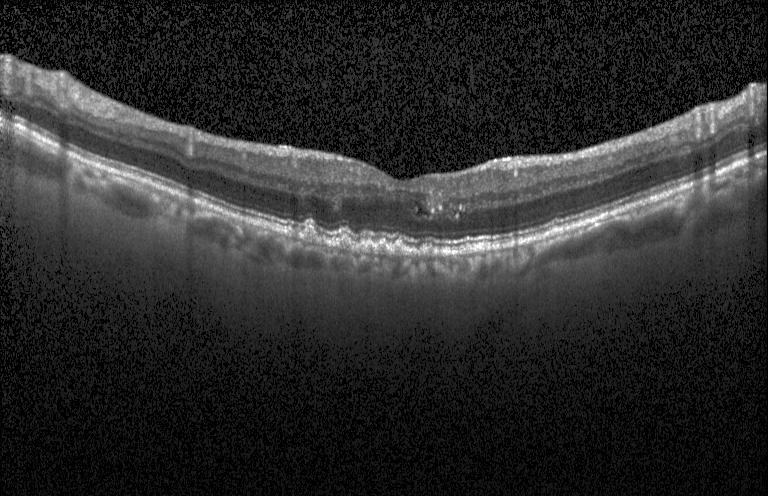 Spectral-domain OCT B-scan: sub-RPE drusenoid deposits.